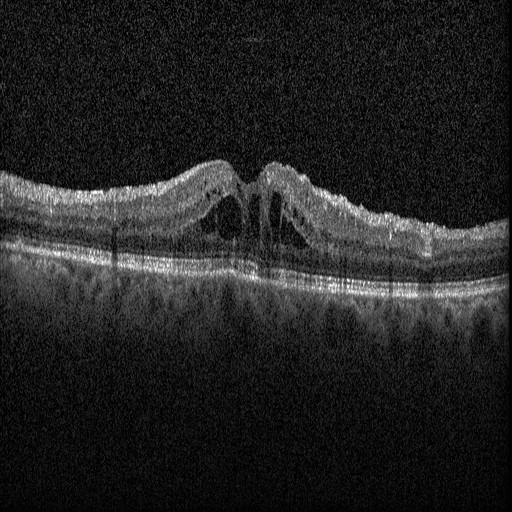
Diagnosis: diabetic macular edema.